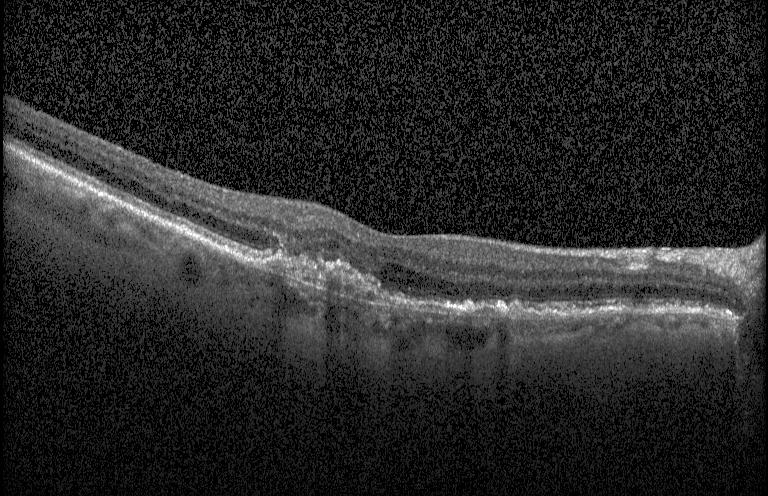
Optical coherence tomography B-scan.
Assessment: a choroidal neovascular membrane.